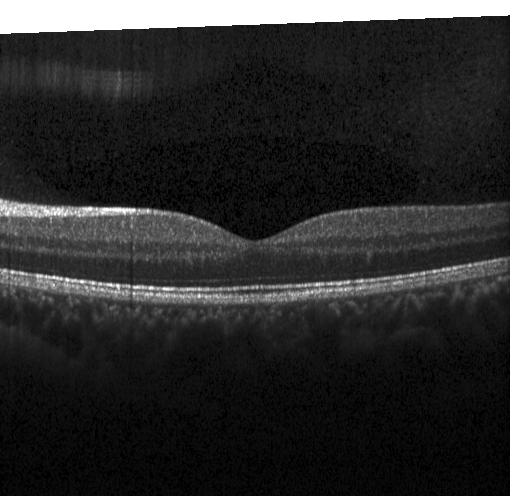

Impression: no evidence of CNV, DME, or drusen.